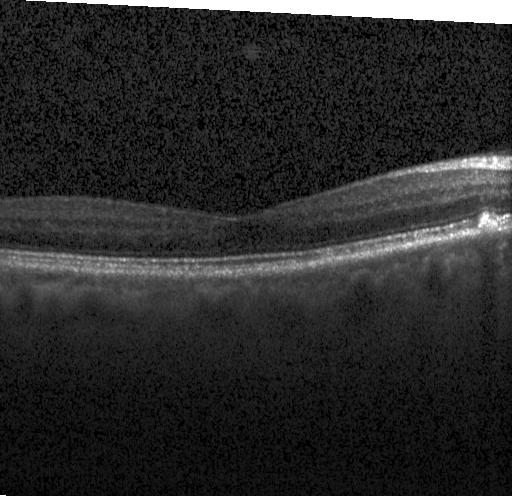
Retinal OCT cross-section.
Diagnosis: sub-RPE drusenoid deposits.